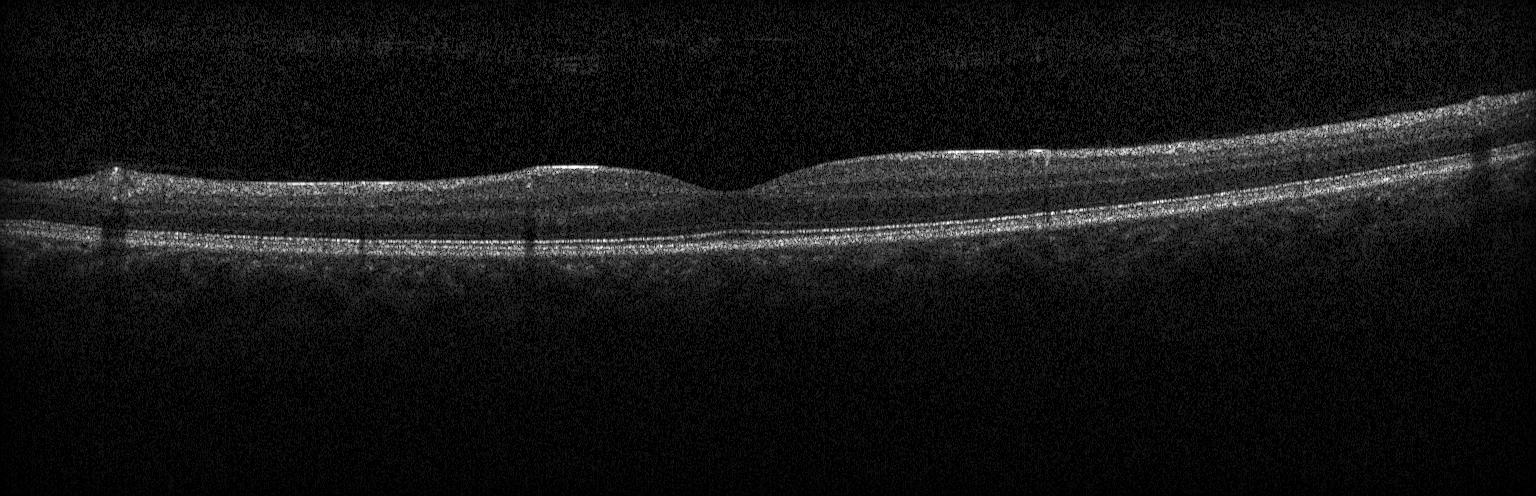
Heidelberg Spectralis; horizontal scan through the fovea; OCT B-scan.
OCT finding: no evidence of choroidal neovascularization, diabetic macular edema, or drusen.